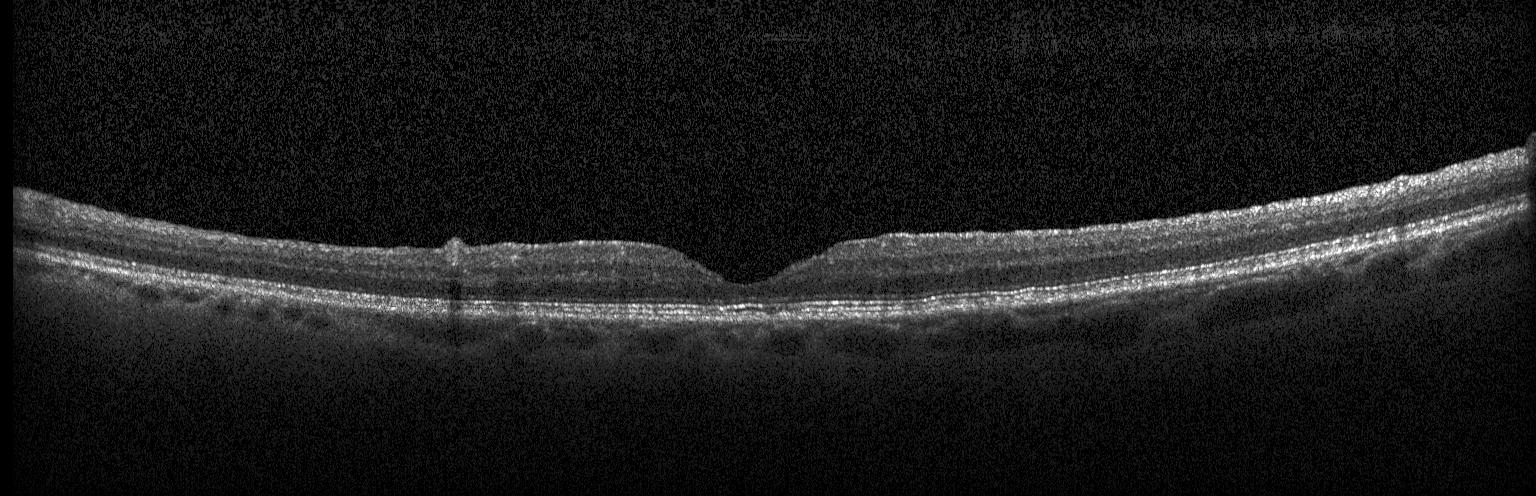 Finding: neither choroidal neovascularization, diabetic macular edema, nor drusen.